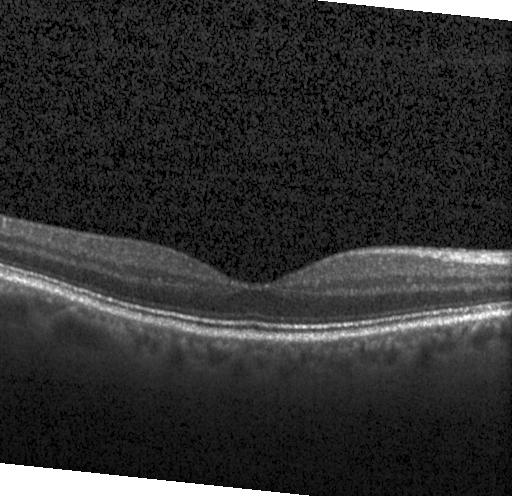 Macular OCT: no choroidal neovascularization, no diabetic macular edema, and no drusen.